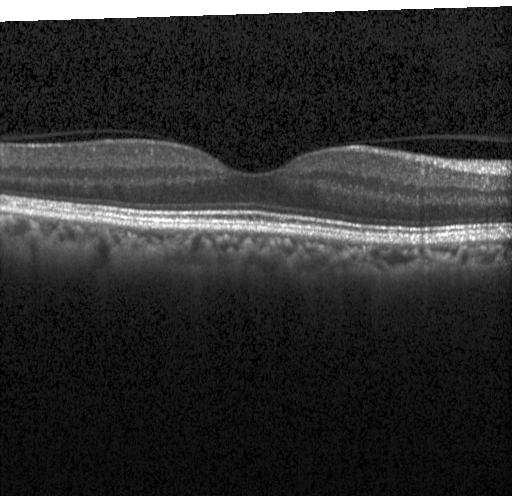 Spectral-domain OCT · acquired on a Heidelberg Spectralis · horizontal scan through the fovea · optical coherence tomography scan — No CNV, no DME, and no drusen.